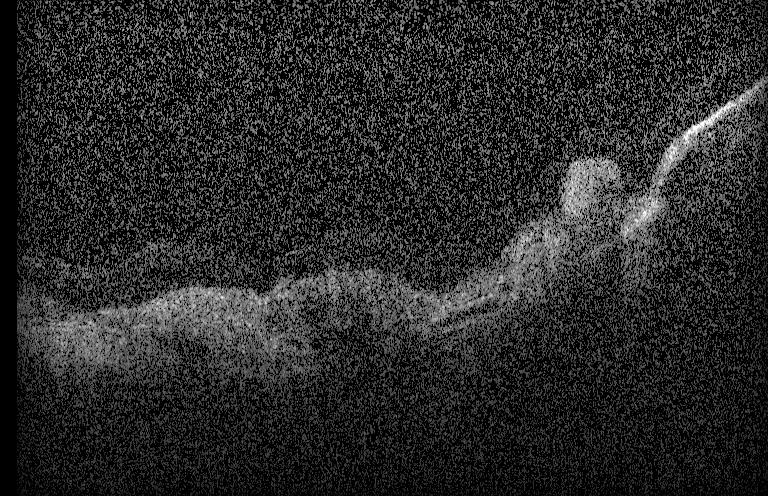 Spectral-domain OCT B-scan: a choroidal neovascular membrane.